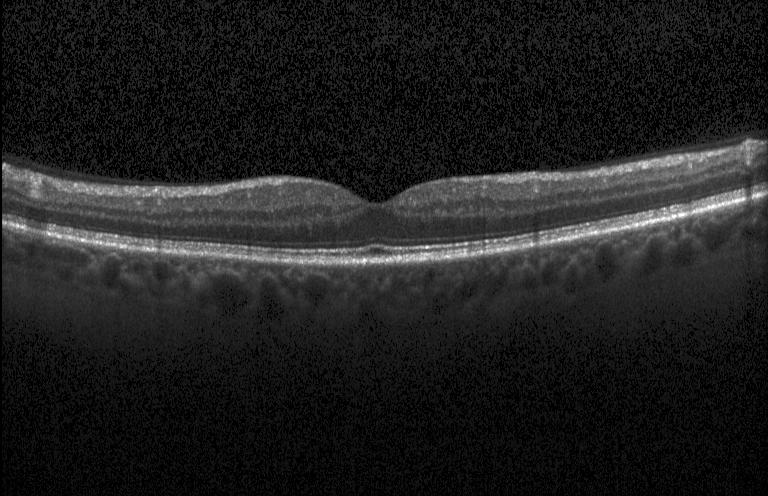
Retinal OCT B-scan — Macular OCT: neither choroidal neovascularization, diabetic macular edema, nor drusen.